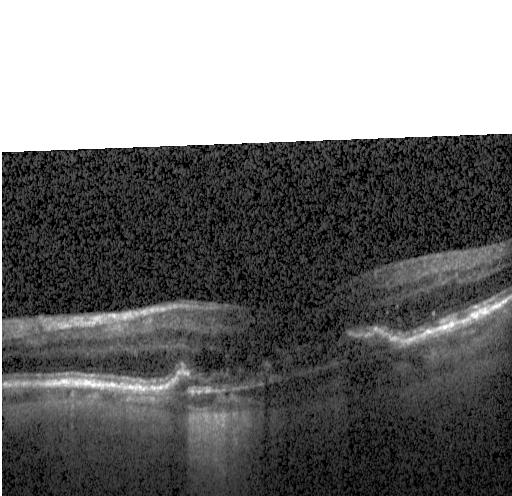 Diagnosis: a choroidal neovascular membrane.